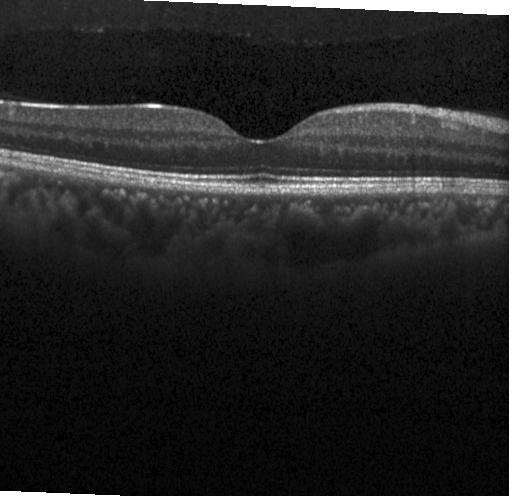

OCT B-scan
Assessment: neither CNV, DME, nor drusen.